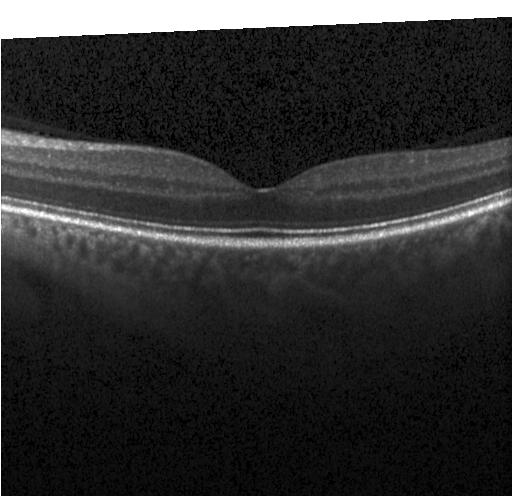 OCT line scan. Instrument: Heidelberg Spectralis — Assessment: no evidence of choroidal neovascularization, diabetic macular edema, or drusen.